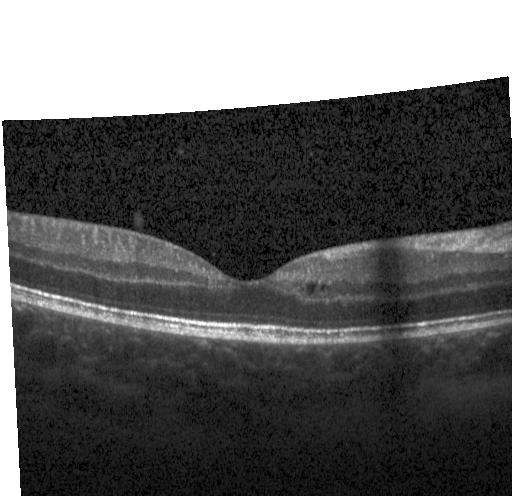

Acquired on a Heidelberg Spectralis, OCT line scan — Impression: diabetic macular edema.